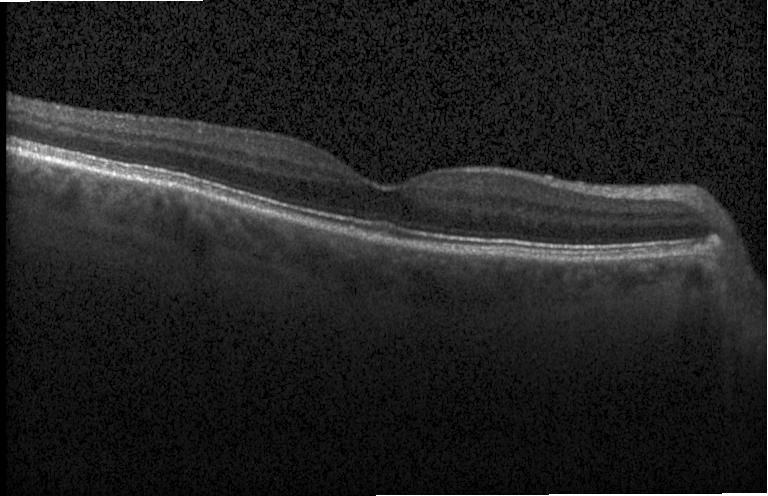

Heidelberg Spectralis. Retinal OCT cross-section. Spectral-domain optical coherence tomography
No CNV, no DME, and no drusen.